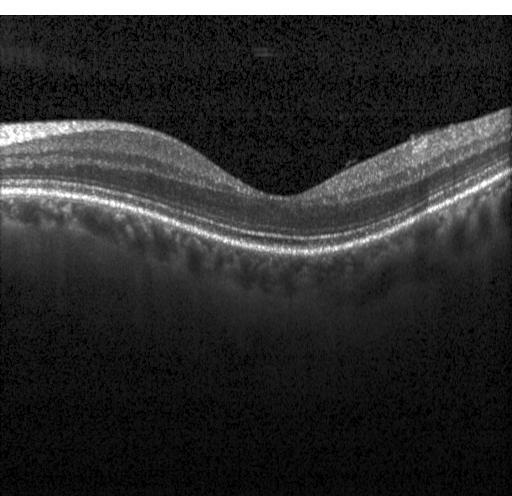 Optical coherence tomography B-scan.
Macular OCT: no evidence of choroidal neovascularization, diabetic macular edema, or drusen.